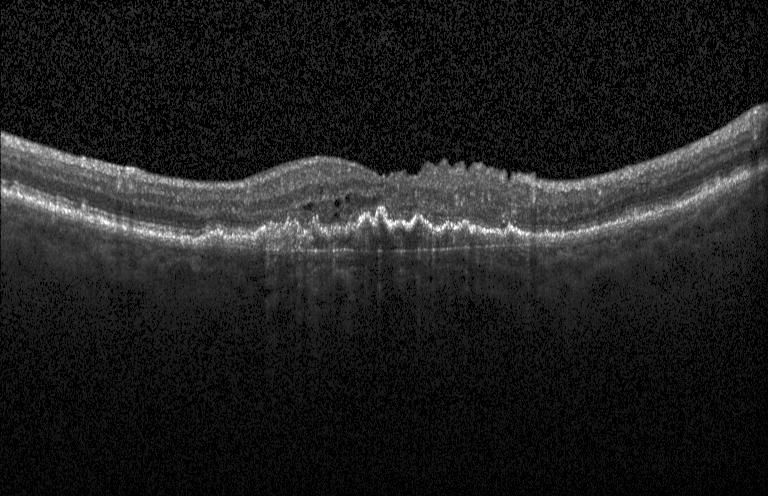 OCT B-scan
Macular OCT: a choroidal neovascular membrane.